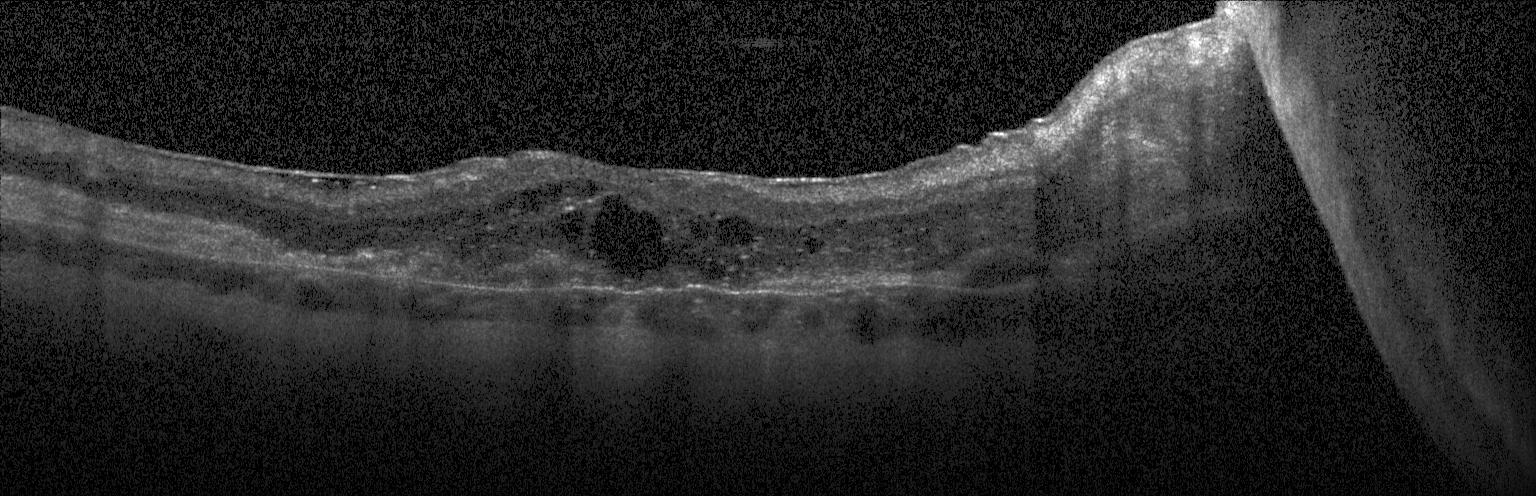
Spectral-domain OCT B-scan: choroidal neovascularization.